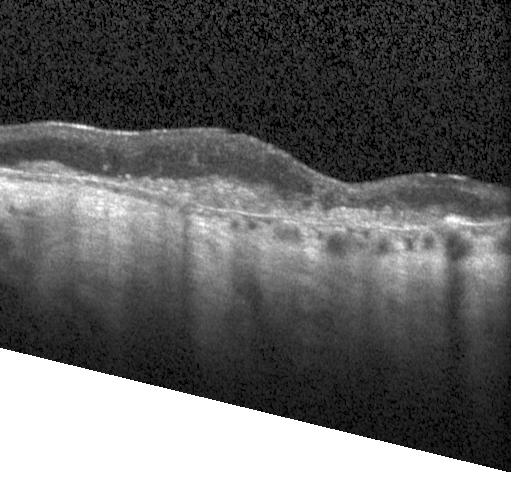

Spectral-domain OCT, OCT line scan, through the macula.
Diagnosis: CNV.